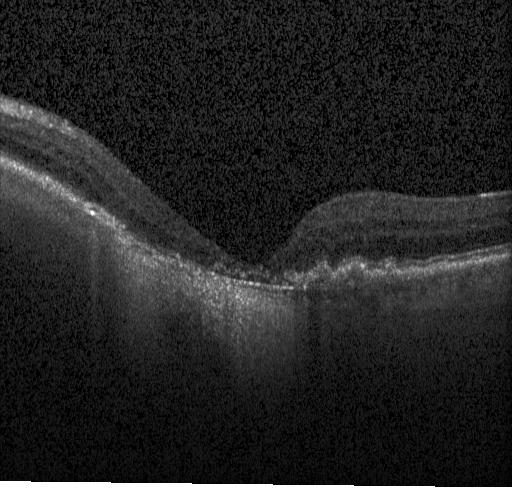

Assessment: a choroidal neovascular membrane.